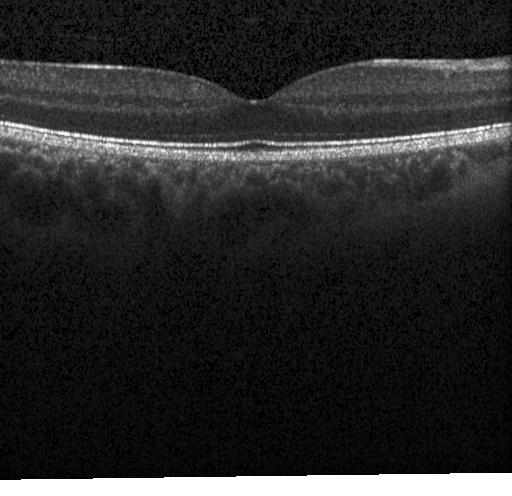 Retinal OCT B-scan · horizontal scan through the fovea · spectral-domain OCT. Impression: neither choroidal neovascularization, diabetic macular edema, nor drusen.